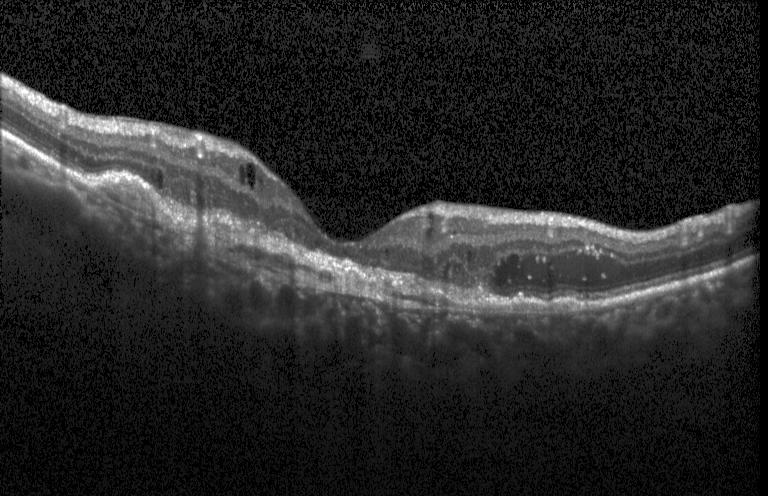 OCT finding: a choroidal neovascular membrane.